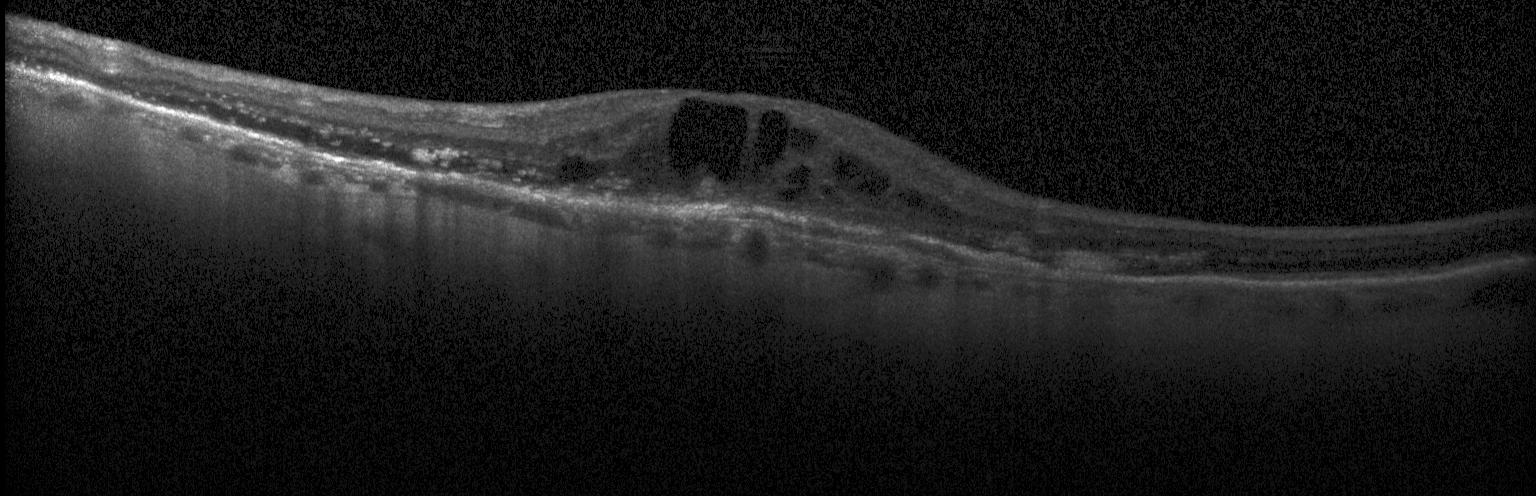

Optical coherence tomography B-scan · spectral-domain optical coherence tomography · Heidelberg Spectralis OCT system · fovea-centered. Assessment: CNV.